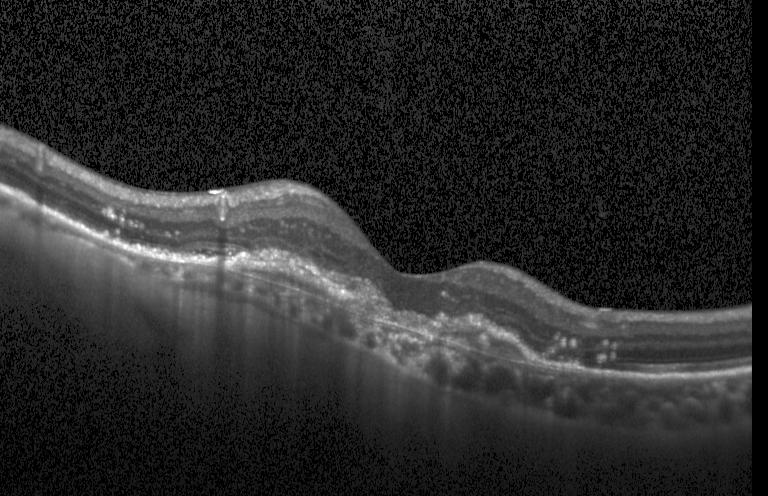
Diagnosis: a choroidal neovascular membrane.